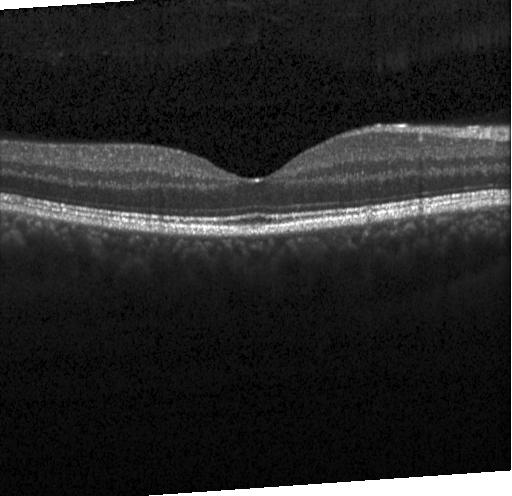 Diagnosis: neither choroidal neovascularization, diabetic macular edema, nor drusen.